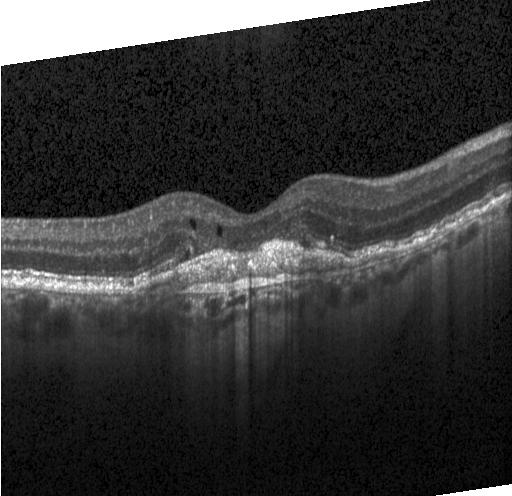 Horizontal scan through the fovea; retinal OCT cross-section; instrument: Heidelberg Spectralis; spectral-domain optical coherence tomography — OCT finding: choroidal neovascularization.